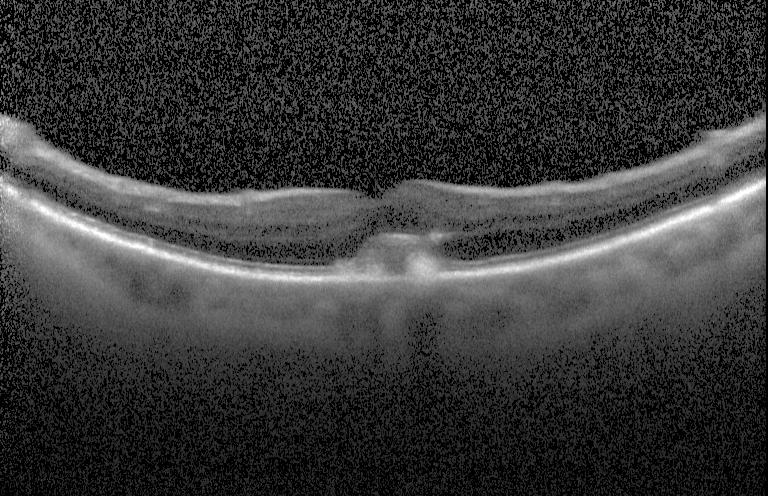

Finding: choroidal neovascularization (CNV).